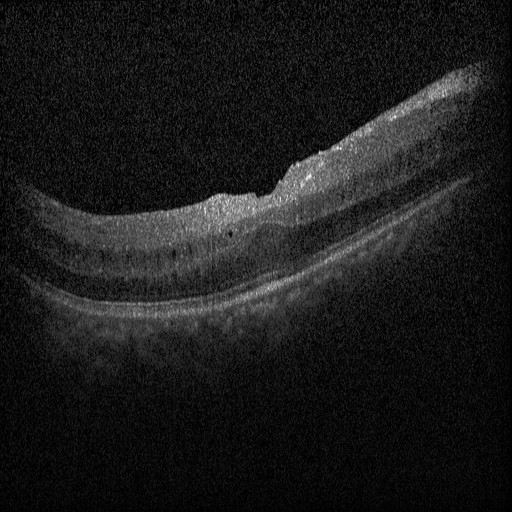 Acquired on a Heidelberg Spectralis, OCT line scan.
Finding: diabetic macular edema (DME).